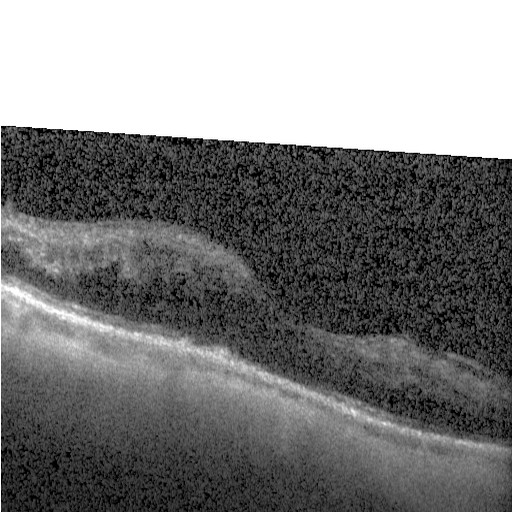

OCT scan showing diabetic macular edema.